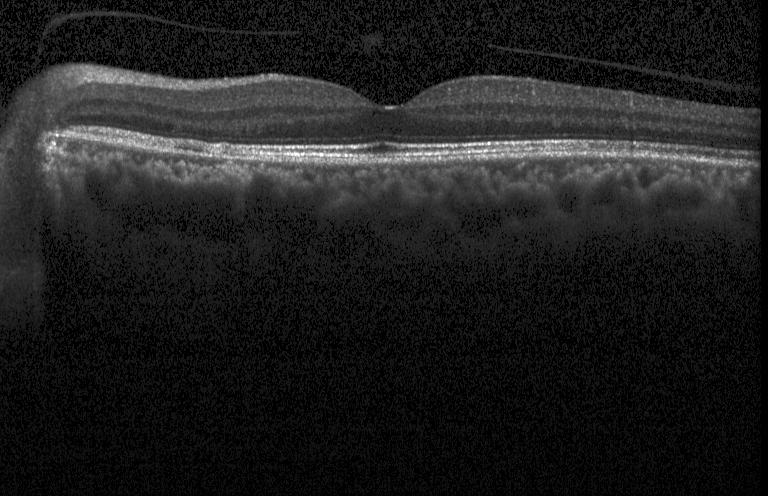 OCT line scan.
Macular OCT: no choroidal neovascularization, diabetic macular edema, or drusen.